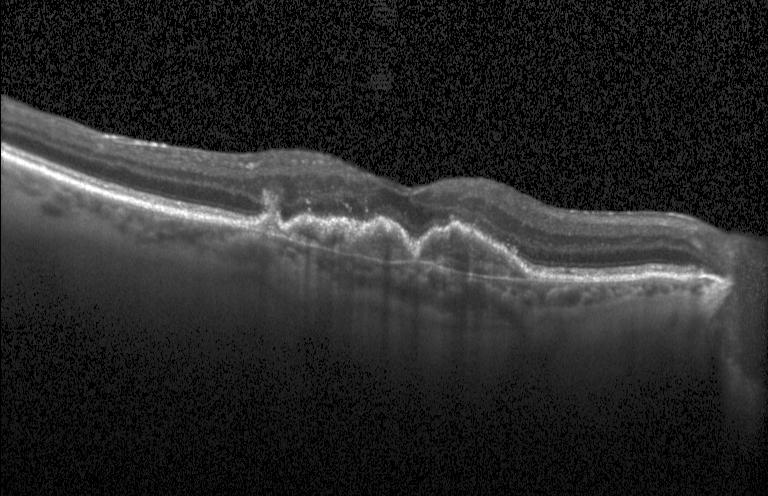 Acquired on a Heidelberg Spectralis, SD-OCT, retinal OCT cross-section, through the macula
Dx: a choroidal neovascular membrane.